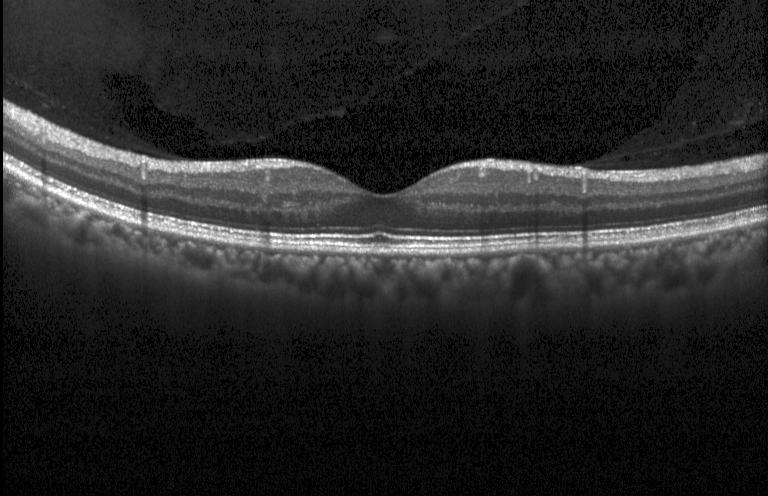
Impression: neither choroidal neovascularization, diabetic macular edema, nor drusen.